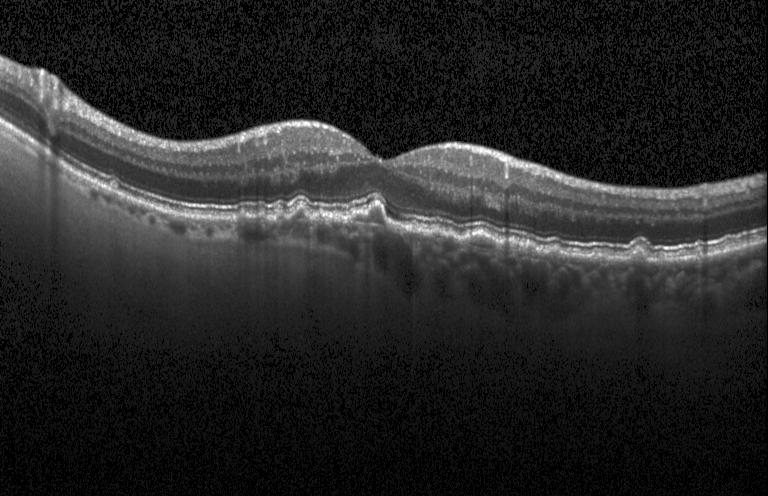 Instrument: Heidelberg Spectralis · horizontal scan through the fovea · retinal OCT cross-section — OCT finding: drusen.